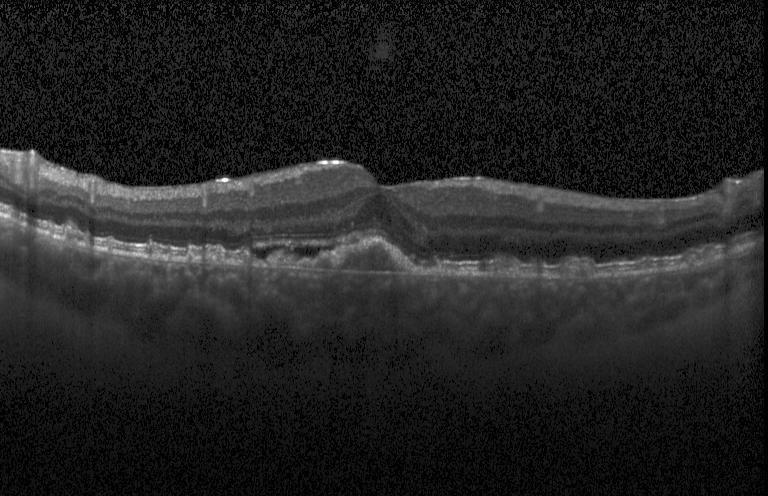 Acquired on a Heidelberg Spectralis; spectral-domain optical coherence tomography; OCT line scan; centered on the fovea — This B-scan demonstrates choroidal neovascularization.